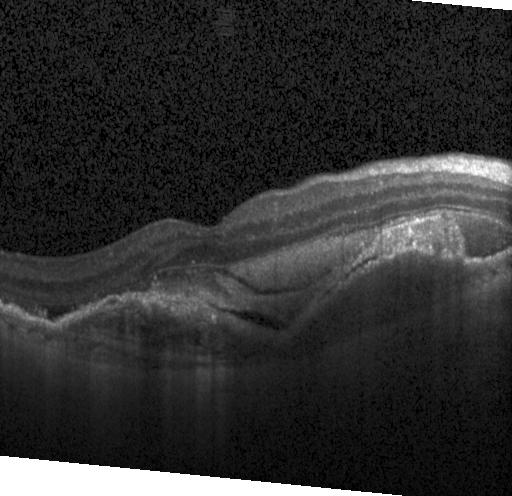
Retinal OCT cross-section. SD-OCT. Heidelberg Spectralis. Centered on the fovea
Impression: CNV.